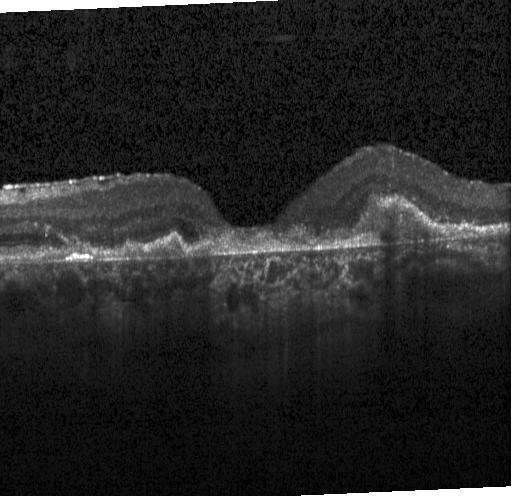 Optical coherence tomography B-scan
OCT finding: a choroidal neovascular membrane.